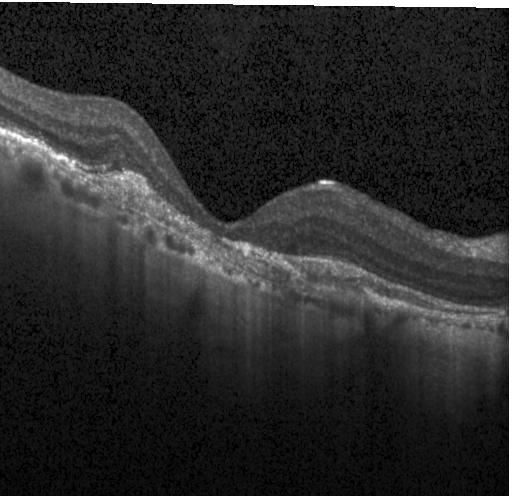
OCT line scan; spectral-domain optical coherence tomography. Impression: a choroidal neovascular membrane.